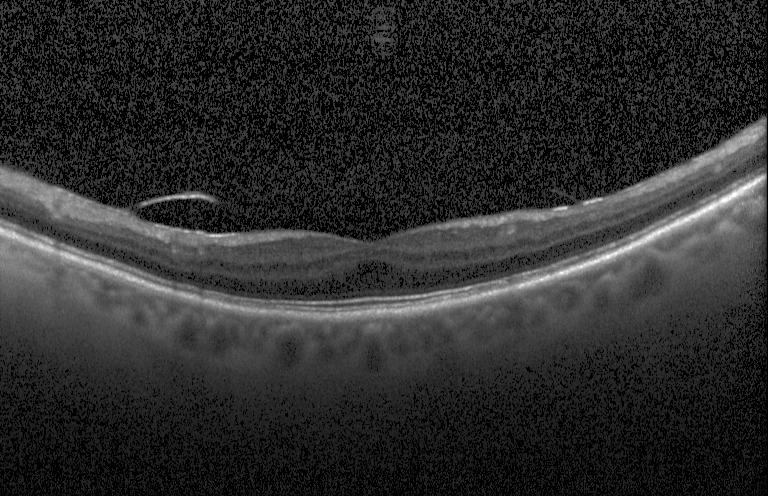
Horizontal scan through the fovea, SD-OCT, OCT B-scan, instrument: Heidelberg Spectralis. Macular OCT: no evidence of CNV, DME, or drusen.